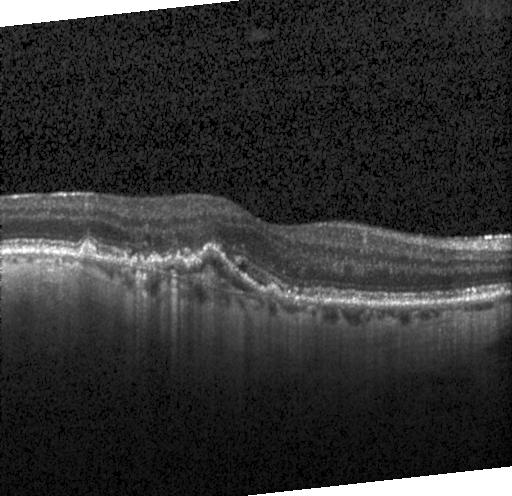 OCT finding: choroidal neovascularization.